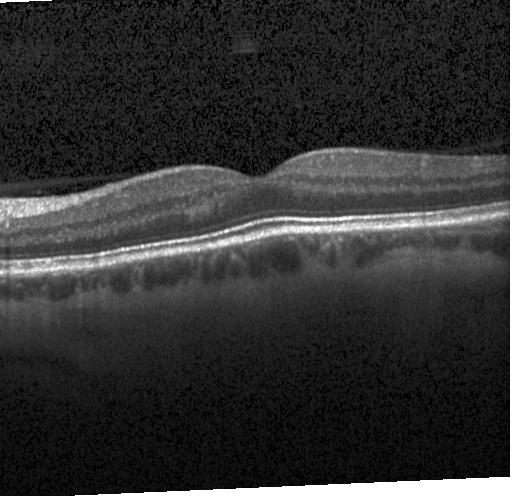 Optical coherence tomography B-scan; instrument: Heidelberg Spectralis.
Impression: no evidence of choroidal neovascularization, diabetic macular edema, or drusen.